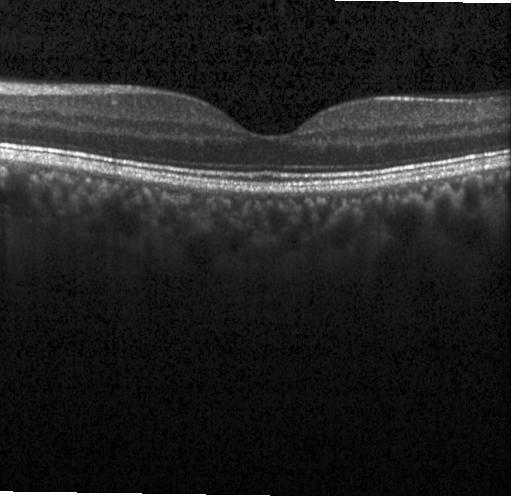 Heidelberg Spectralis. OCT line scan. Through the macula.
Finding: no choroidal neovascularization, diabetic macular edema, or drusen.